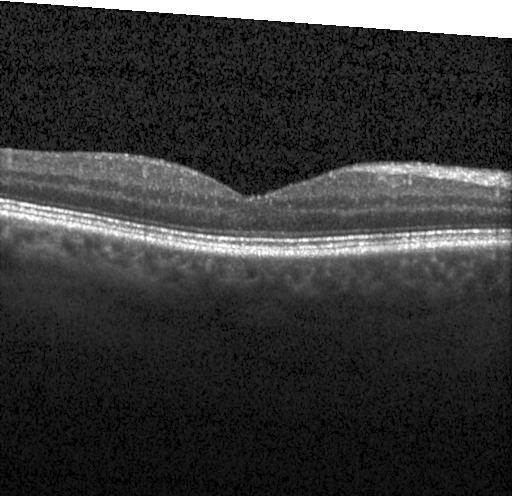 Retinal OCT cross-section; instrument: Heidelberg Spectralis; centered on the fovea; spectral-domain optical coherence tomography
Assessment: no evidence of choroidal neovascularization, diabetic macular edema, or drusen.